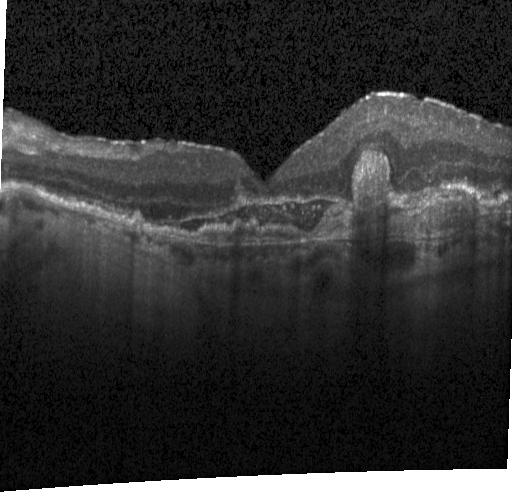
The scan shows a choroidal neovascular membrane.